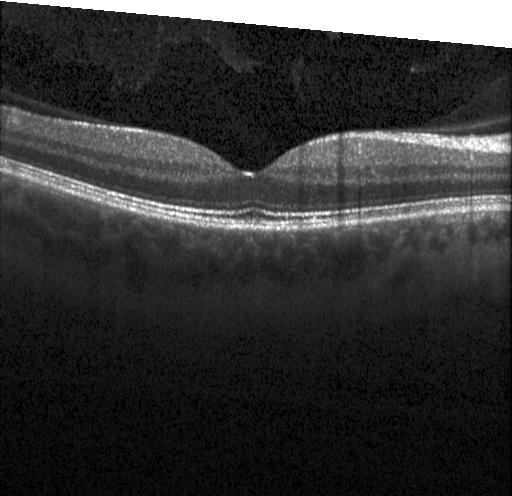
Retinal OCT B-scan — No evidence of choroidal neovascularization, diabetic macular edema, or drusen.